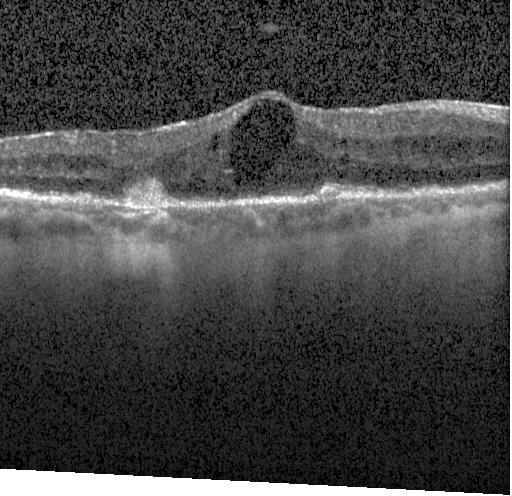 Heidelberg Spectralis OCT system · retinal OCT cross-section · fovea-centered. Finding: choroidal neovascularization.